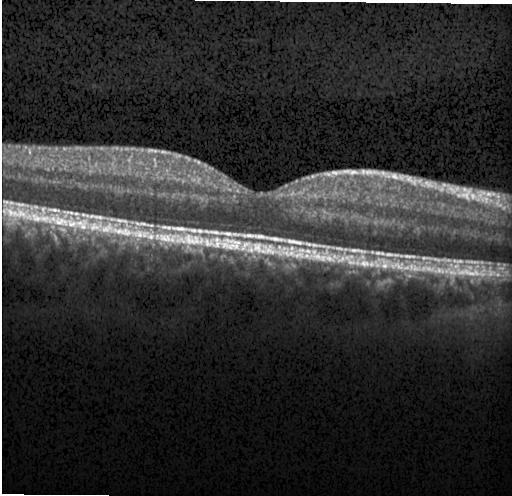 SD-OCT; OCT line scan; Heidelberg Spectralis
Macular OCT: no choroidal neovascularization, diabetic macular edema, or drusen.